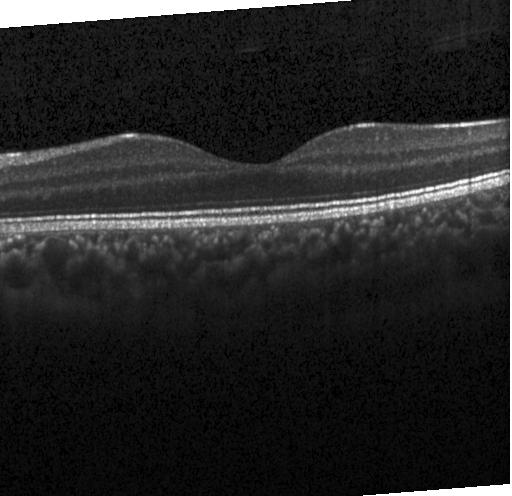

Macular scan, retinal OCT B-scan.
Diagnosis: no CNV, no DME, and no drusen.